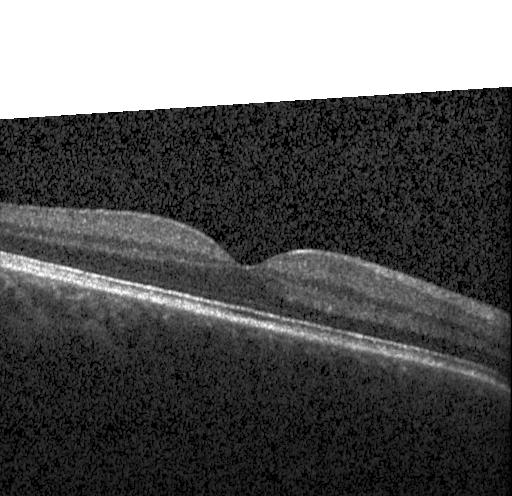 Finding: neither CNV, DME, nor drusen.